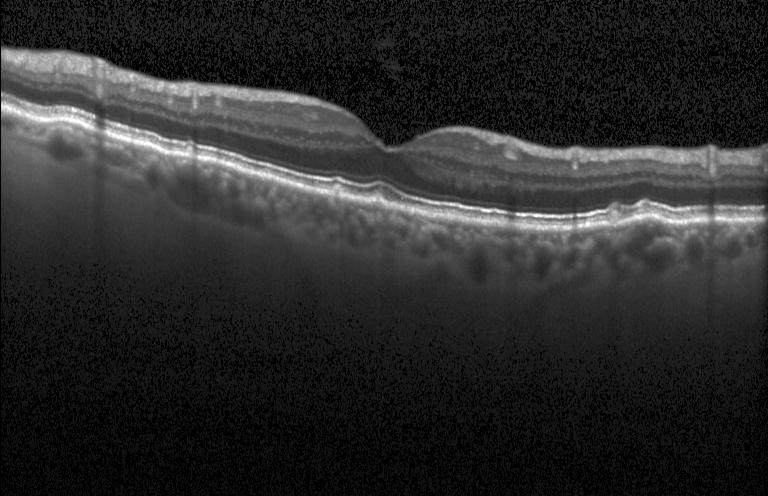 Macular scan · optical coherence tomography scan · Heidelberg Spectralis · SD-OCT.
This B-scan demonstrates drusen.